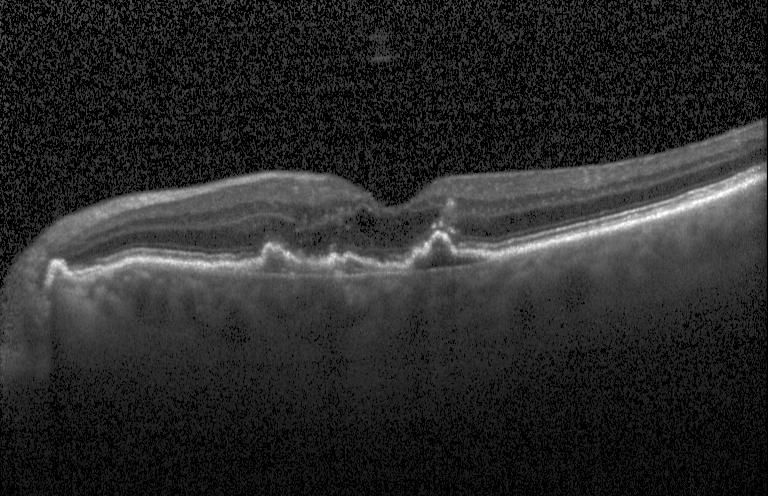

Dx: CNV.